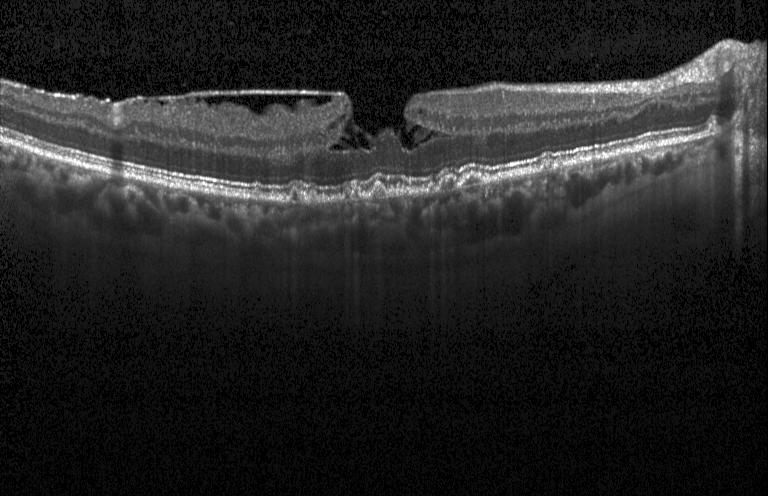

Macular OCT demonstrating multiple drusen.